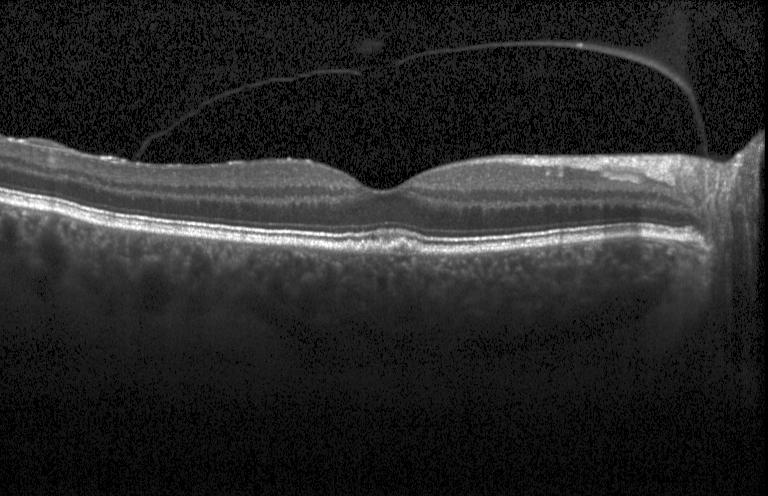 This B-scan demonstrates multiple drusen.